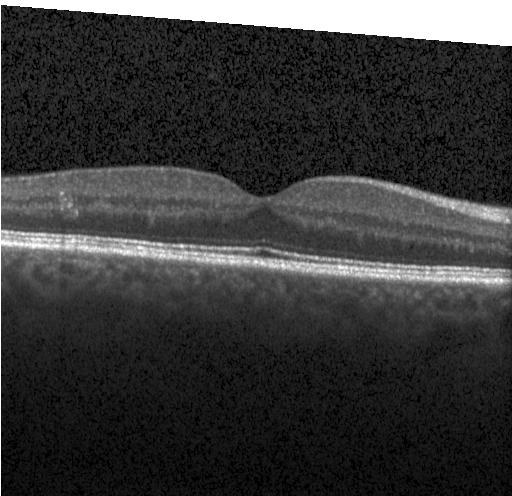
OCT scan showing no evidence of CNV, DME, or drusen.